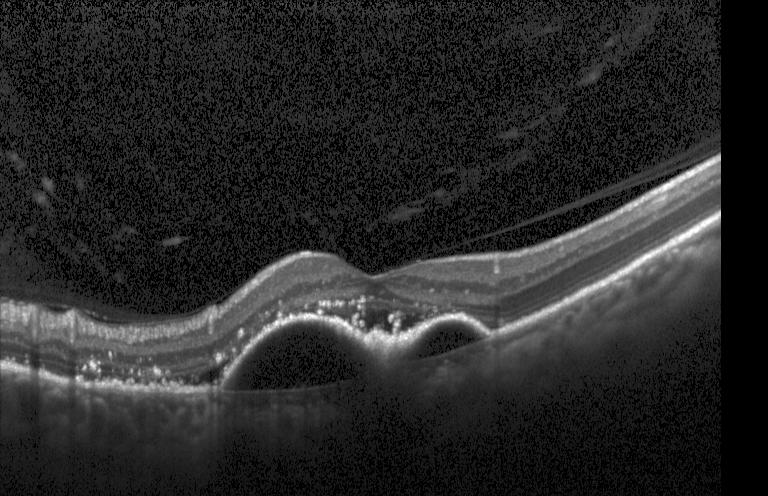

Optical coherence tomography B-scan. Spectral-domain OCT. Instrument: Heidelberg Spectralis. Macular scan. Impression: choroidal neovascularization.